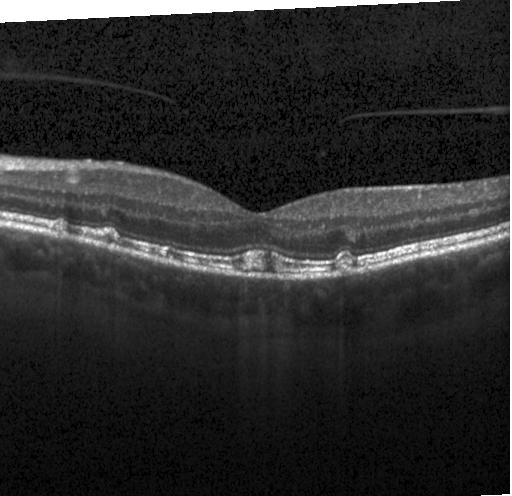
Fovea-centered · instrument: Heidelberg Spectralis · OCT line scan · SD-OCT. Diagnosis: multiple drusen.